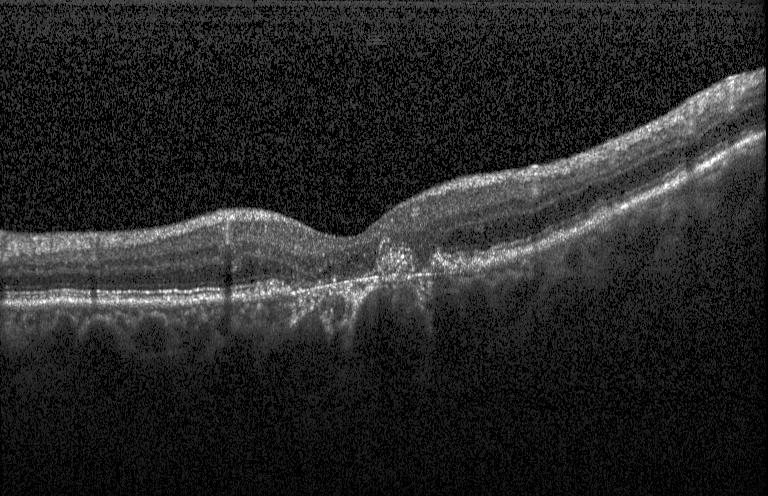

Macular scan, OCT B-scan, Heidelberg Spectralis, spectral-domain optical coherence tomography — Impression: a choroidal neovascular membrane.